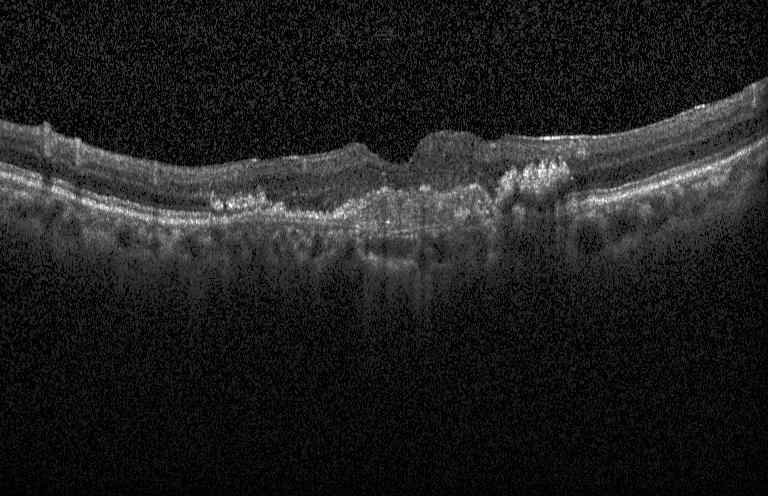
Macular OCT demonstrating a choroidal neovascular membrane.